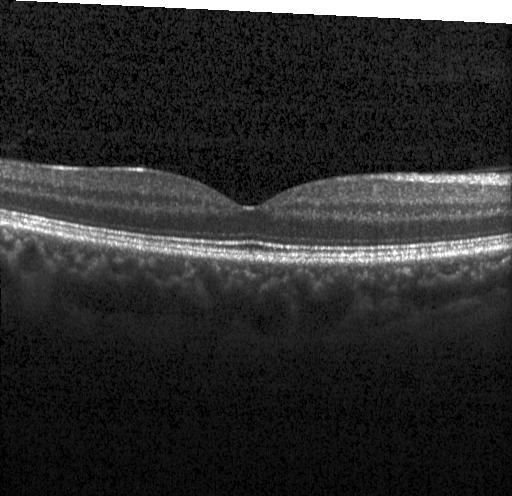
OCT B-scan showing no evidence of choroidal neovascularization, diabetic macular edema, or drusen.